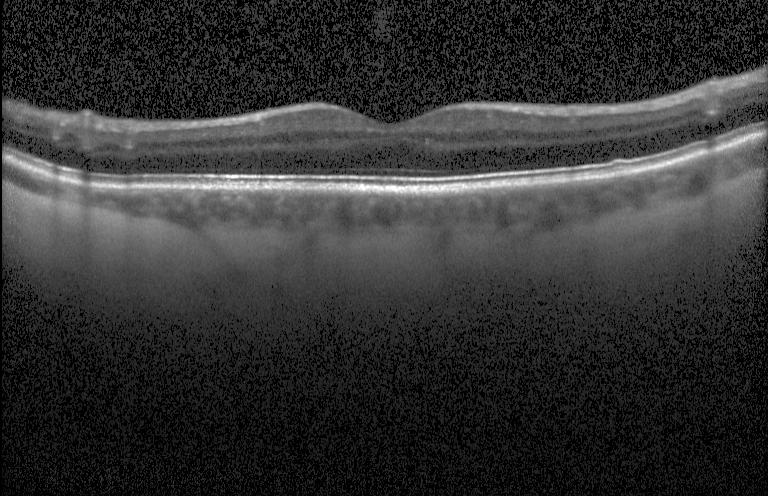 Spectral-domain optical coherence tomography, optical coherence tomography B-scan — Macular OCT: no choroidal neovascularization, no diabetic macular edema, and no drusen.